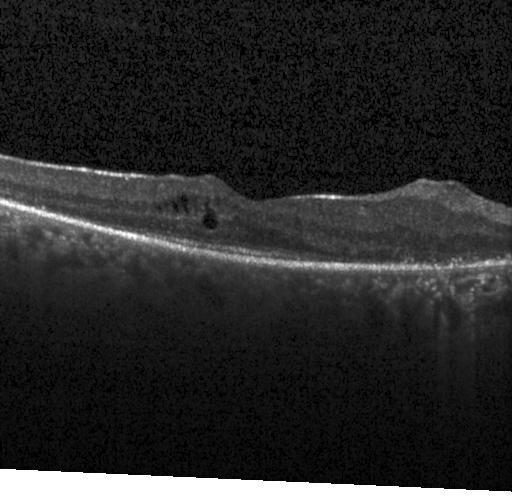
Fovea-centered · instrument: Heidelberg Spectralis · spectral-domain optical coherence tomography · optical coherence tomography scan. Macular OCT: diabetic macular edema (DME).